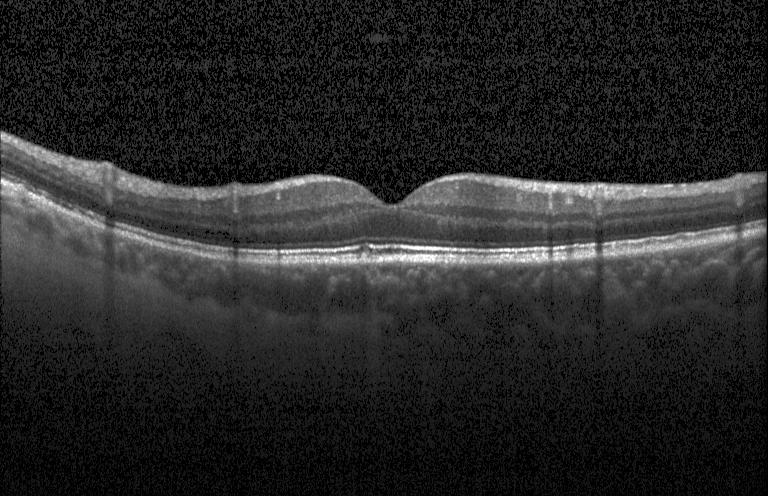
Impression: neither CNV, DME, nor drusen.